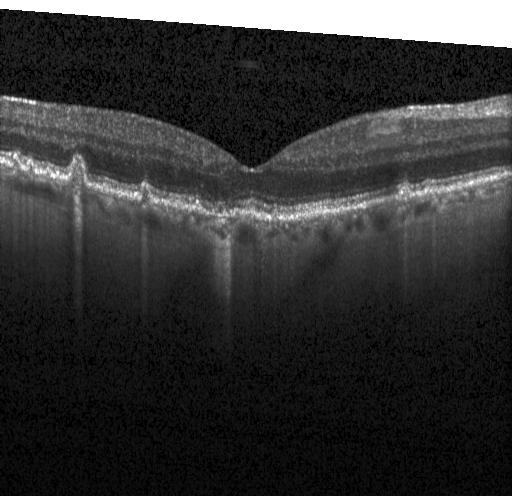 OCT B-scan showing drusen.